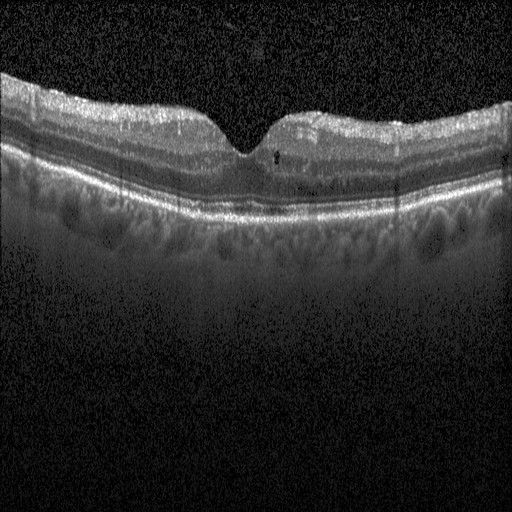
Macular scan; OCT B-scan.
This B-scan demonstrates diabetic macular edema (DME).